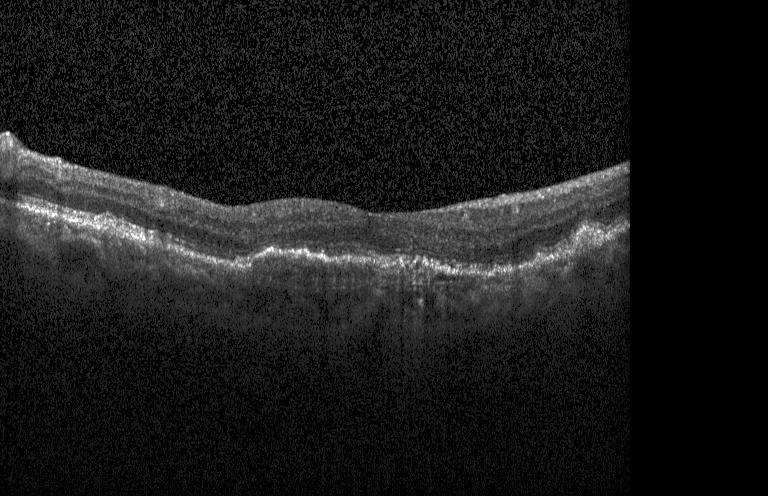

Acquired on a Heidelberg Spectralis · retinal OCT cross-section · SD-OCT
This B-scan demonstrates choroidal neovascularization.